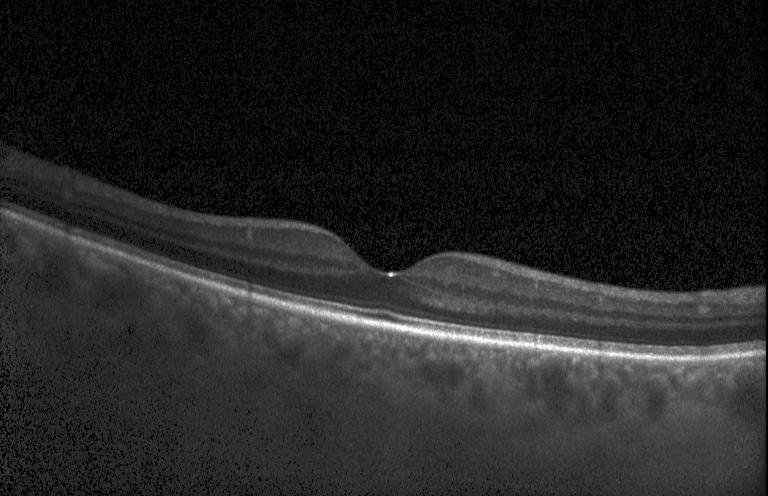 Acquired on a Heidelberg Spectralis. OCT line scan — Diagnosis: no choroidal neovascularization, diabetic macular edema, or drusen.